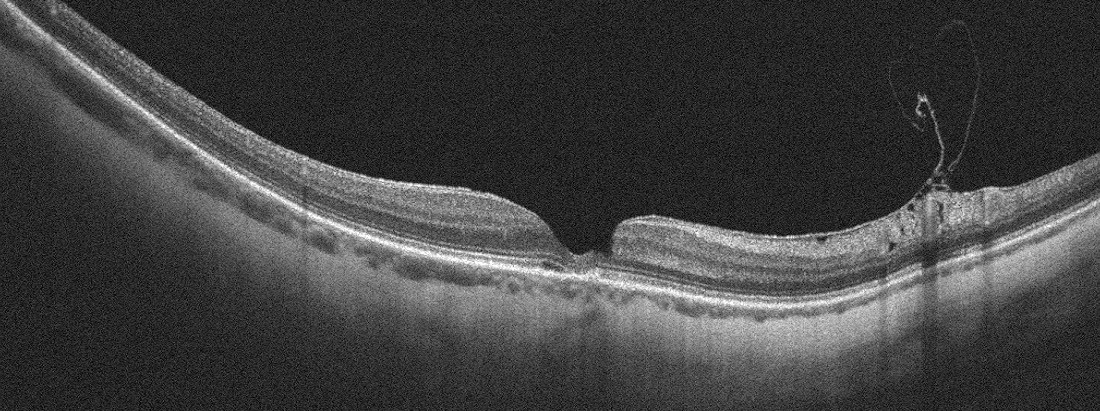 Fovea-centered; optical coherence tomography scan; acquired on an Optovue Avanti RTVue XR.
Impression: epiretinal membrane.